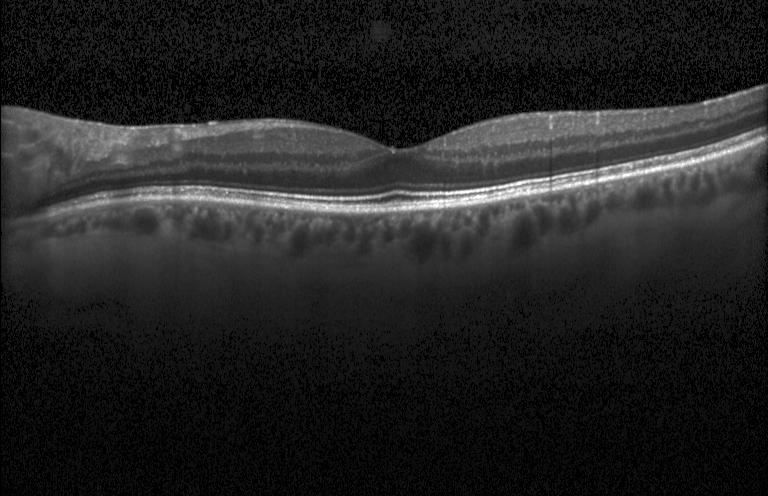 Impression: neither choroidal neovascularization, diabetic macular edema, nor drusen.